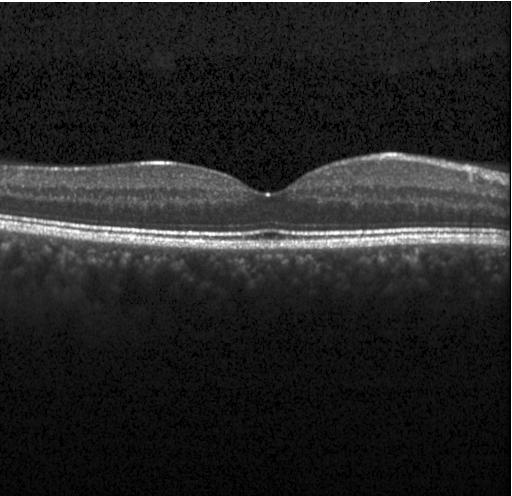

Diagnosis: no evidence of CNV, DME, or drusen.